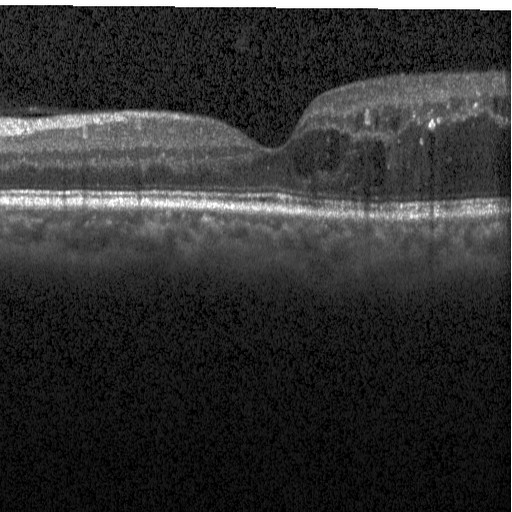 Diabetic macular edema.